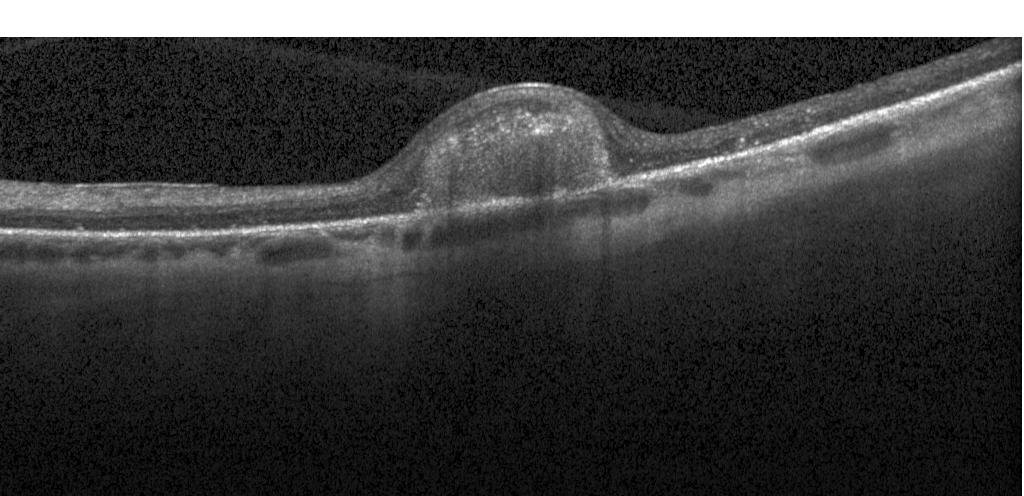

Diagnosis: choroidal neovascularization.